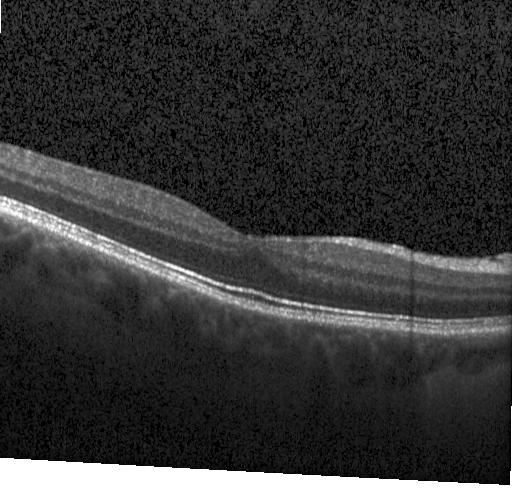

Finding: no evidence of choroidal neovascularization, diabetic macular edema, or drusen.